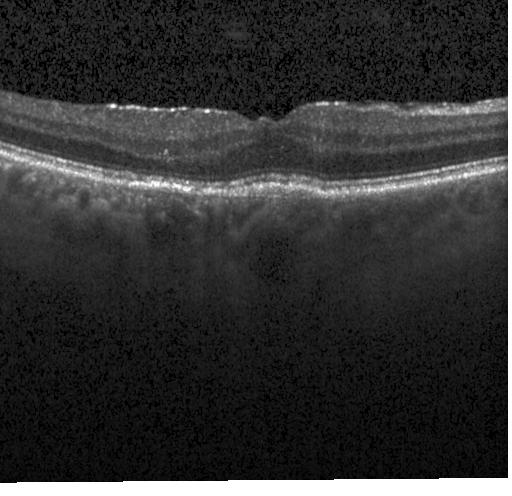
Retinal OCT B-scan. Finding: a choroidal neovascular membrane.